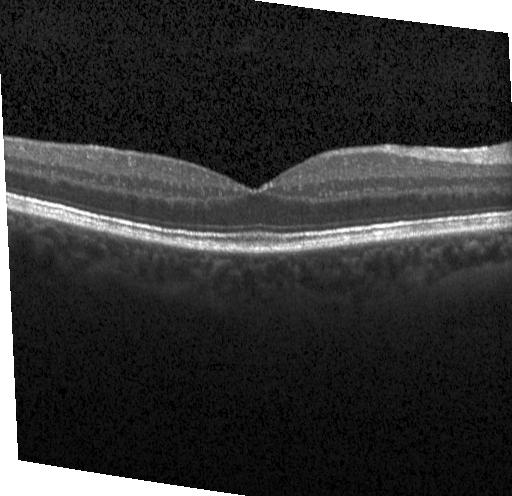
Finding: no CNV, no DME, and no drusen.